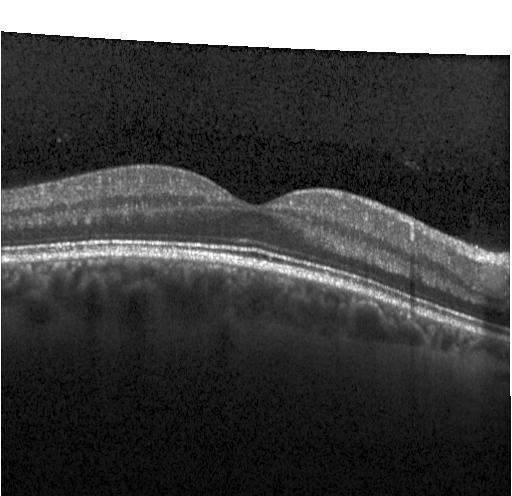

OCT scan showing no choroidal neovascularization, diabetic macular edema, or drusen.